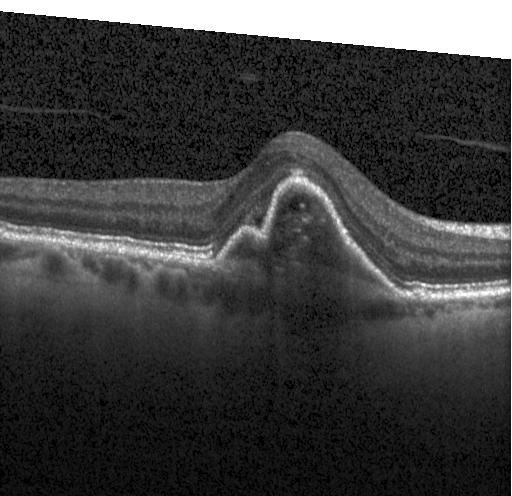

Impression: choroidal neovascularization (CNV).